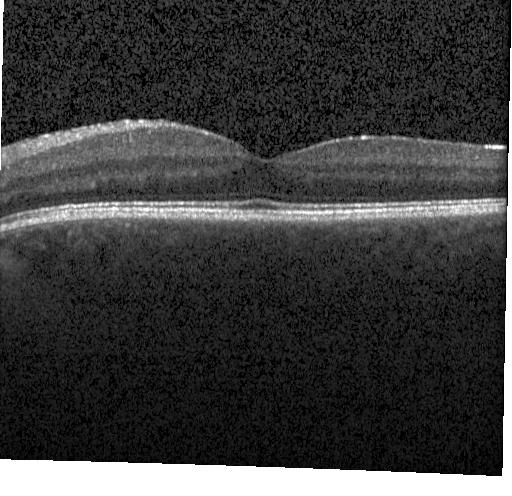 Macular OCT: no evidence of CNV, DME, or drusen.